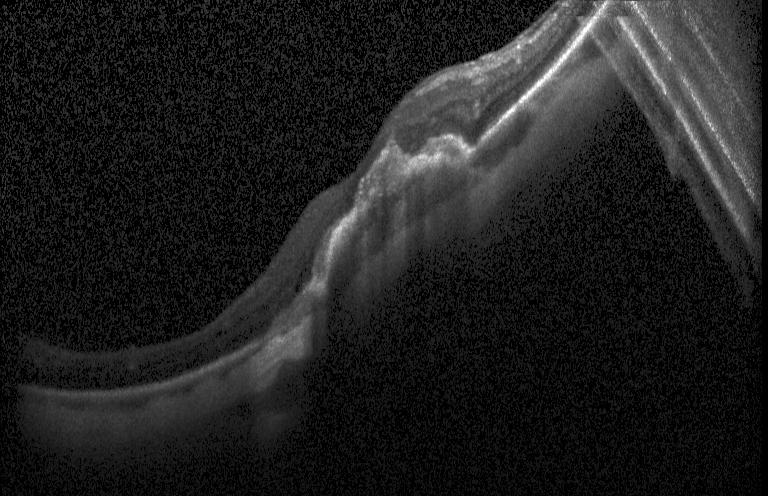
Macular scan; OCT B-scan
Diagnosis: choroidal neovascularization (CNV).